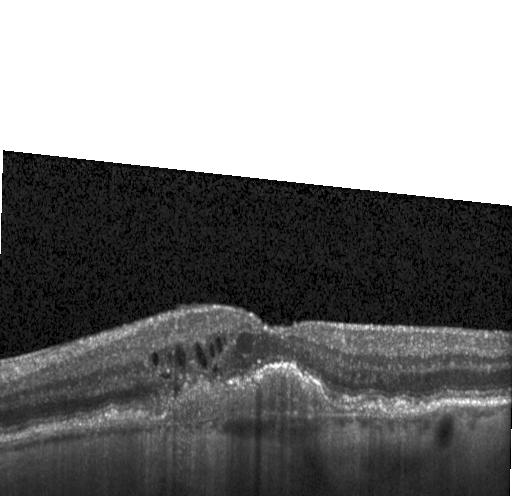
OCT line scan — Dx: CNV.